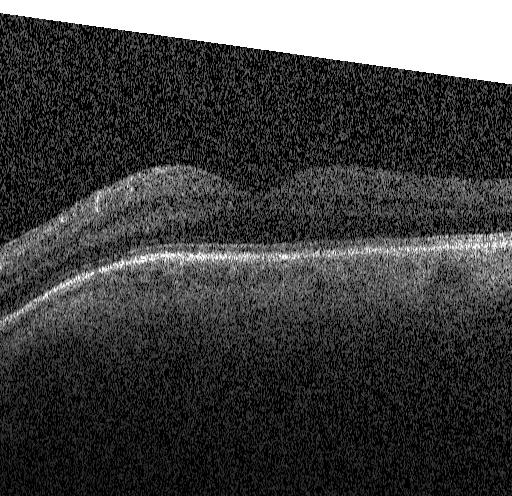
Retinal OCT cross-section.
No evidence of choroidal neovascularization, diabetic macular edema, or drusen.